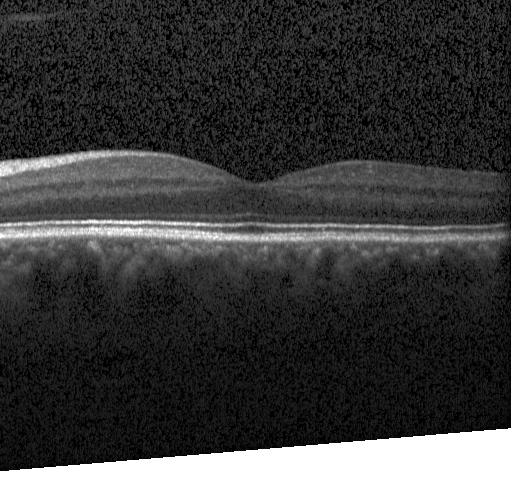
Retinal OCT B-scan
Finding: no choroidal neovascularization, diabetic macular edema, or drusen.